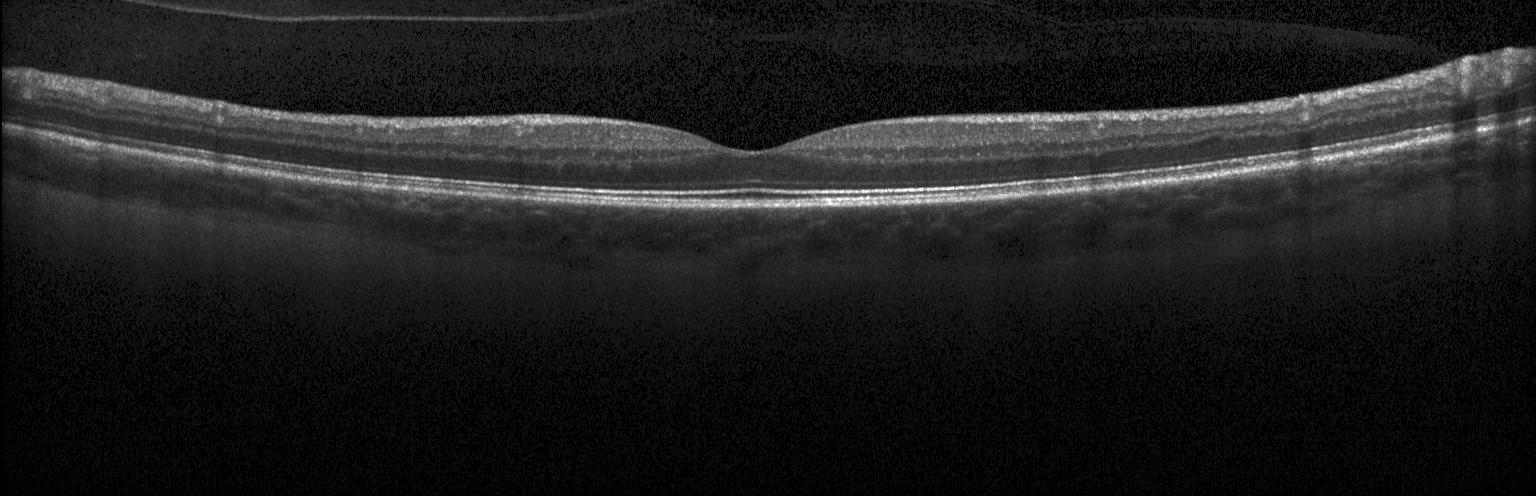

Retinal OCT cross-section. No choroidal neovascularization, diabetic macular edema, or drusen.